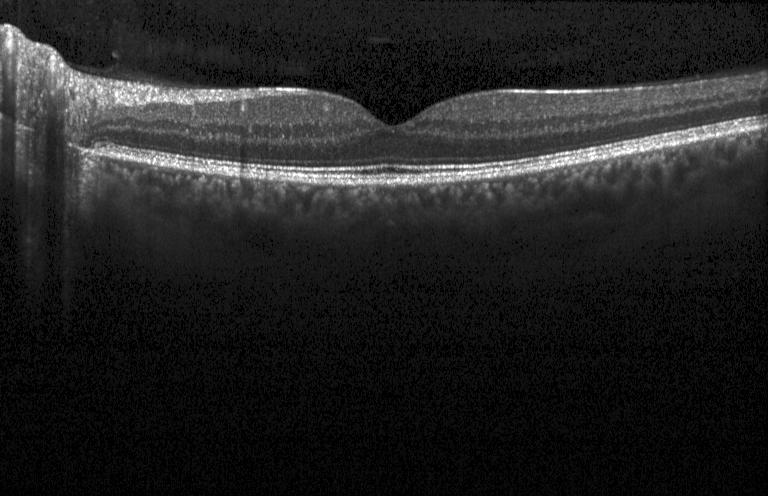

Heidelberg Spectralis OCT system. OCT line scan. Spectral-domain OCT. Macular scan
Assessment: no choroidal neovascularization, no diabetic macular edema, and no drusen.